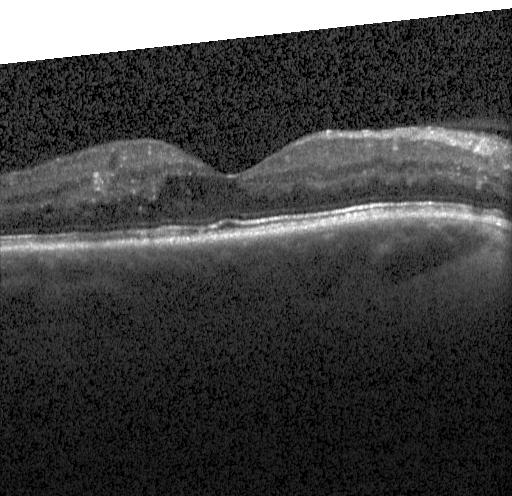

This B-scan demonstrates diabetic macular edema (DME).